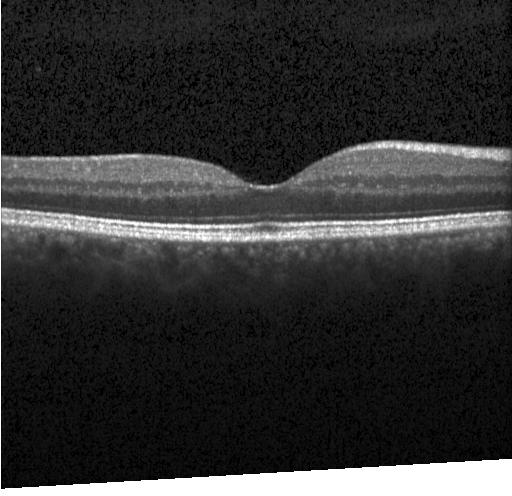 Retinal OCT B-scan. Instrument: Heidelberg Spectralis. Centered on the fovea. Spectral-domain optical coherence tomography.
OCT finding: no evidence of choroidal neovascularization, diabetic macular edema, or drusen.